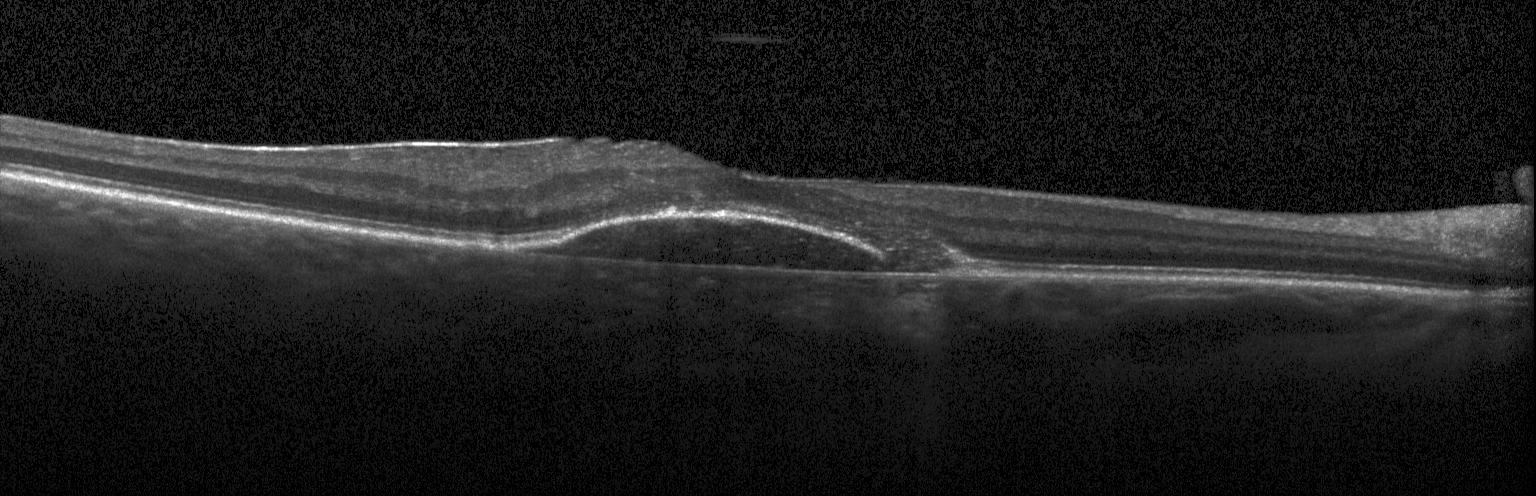 Retinal OCT cross-section · spectral-domain OCT · horizontal scan through the fovea — Impression: a choroidal neovascular membrane.